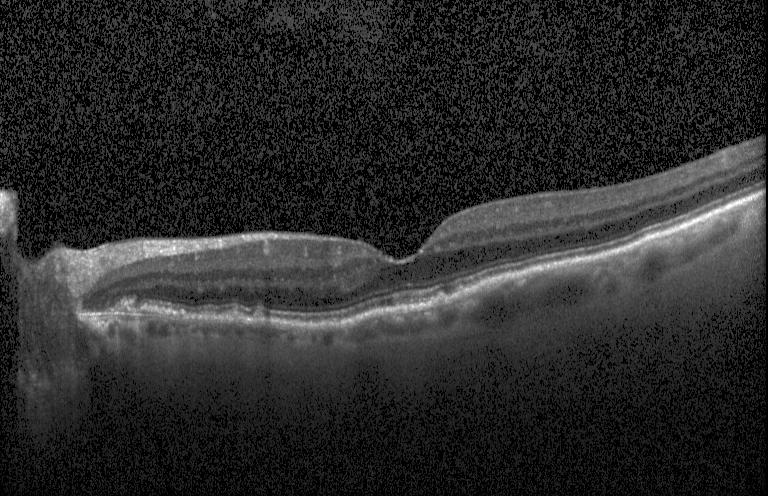 Retinal OCT cross-section. Horizontal scan through the fovea. Heidelberg Spectralis. Spectral-domain optical coherence tomography.
Impression: multiple drusen.